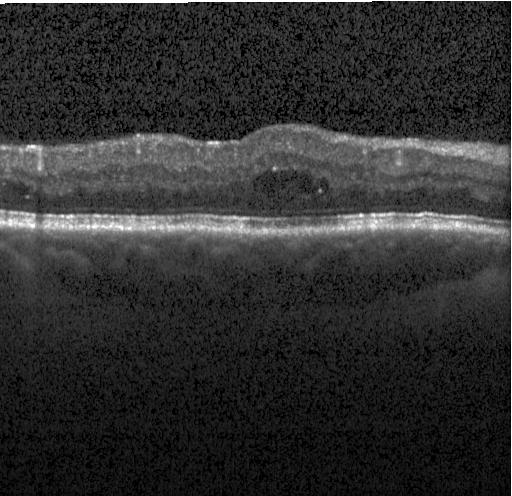
Finding: diabetic macular edema.